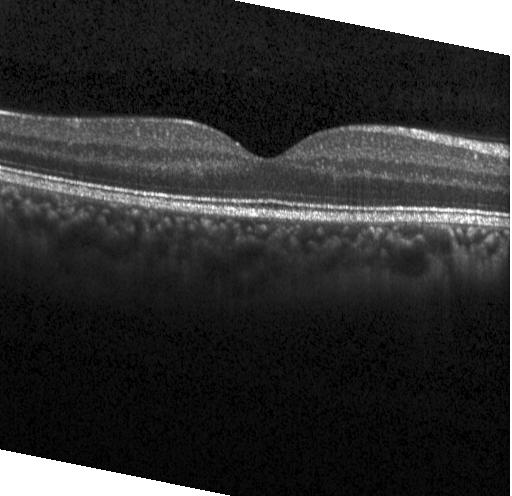 Dx: neither choroidal neovascularization, diabetic macular edema, nor drusen.